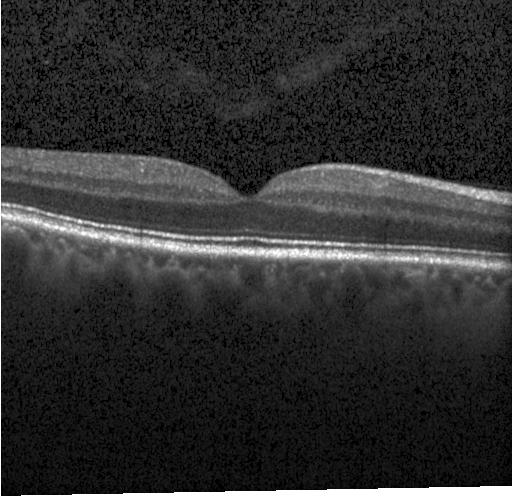 Retinal OCT B-scan. Finding: no evidence of choroidal neovascularization, diabetic macular edema, or drusen.